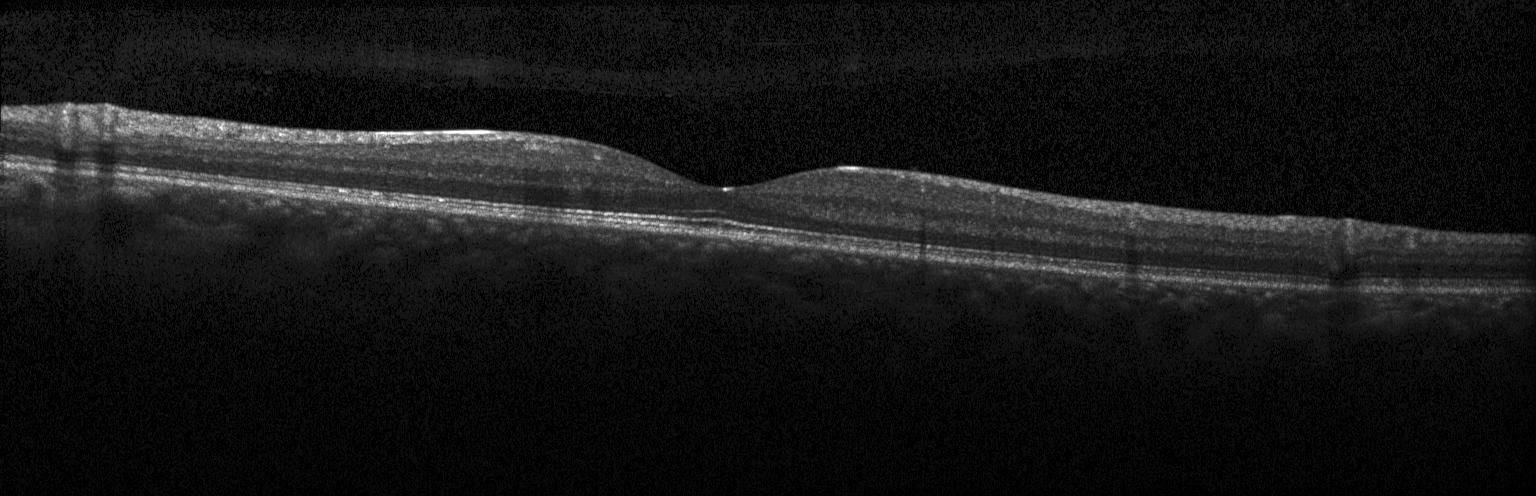 Optical coherence tomography B-scan
Diagnosis: neither choroidal neovascularization, diabetic macular edema, nor drusen.